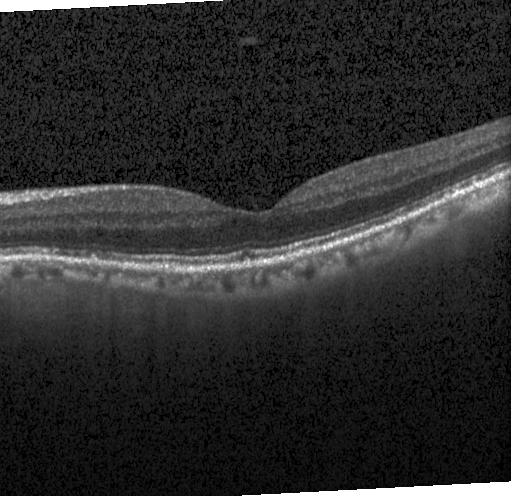
OCT line scan; Heidelberg Spectralis OCT system.
This B-scan demonstrates no choroidal neovascularization, diabetic macular edema, or drusen.